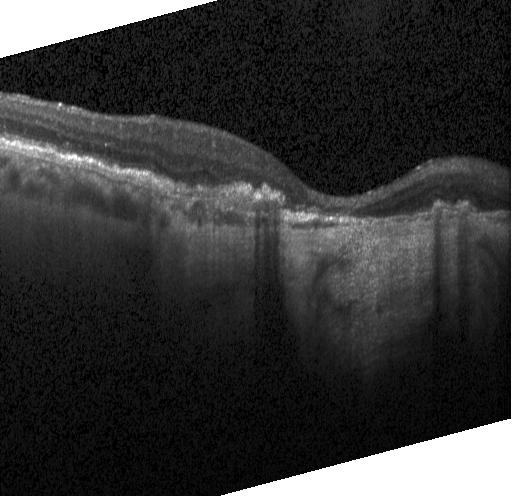

OCT B-scan.
The scan shows choroidal neovascularization (CNV).